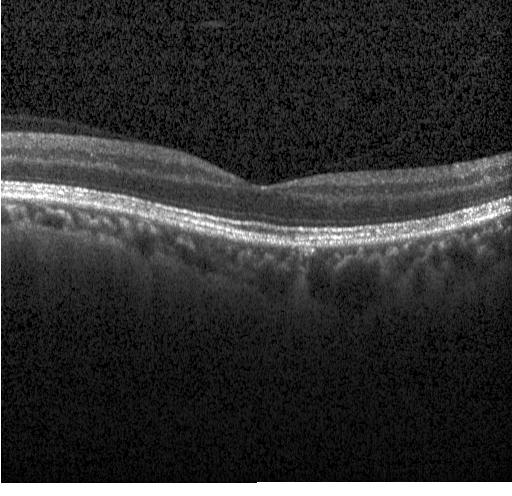 This B-scan demonstrates no choroidal neovascularization, no diabetic macular edema, and no drusen.